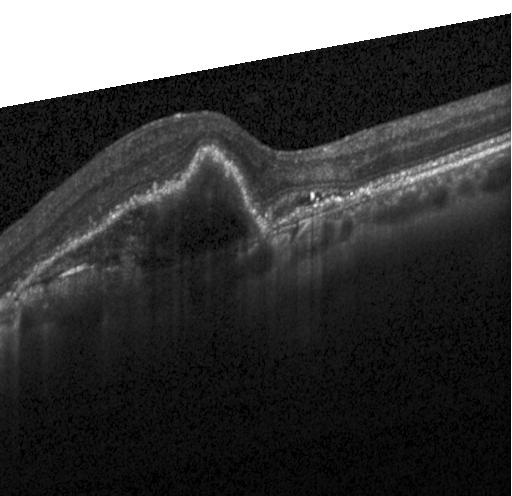

Optical coherence tomography scan
Dx: a choroidal neovascular membrane.